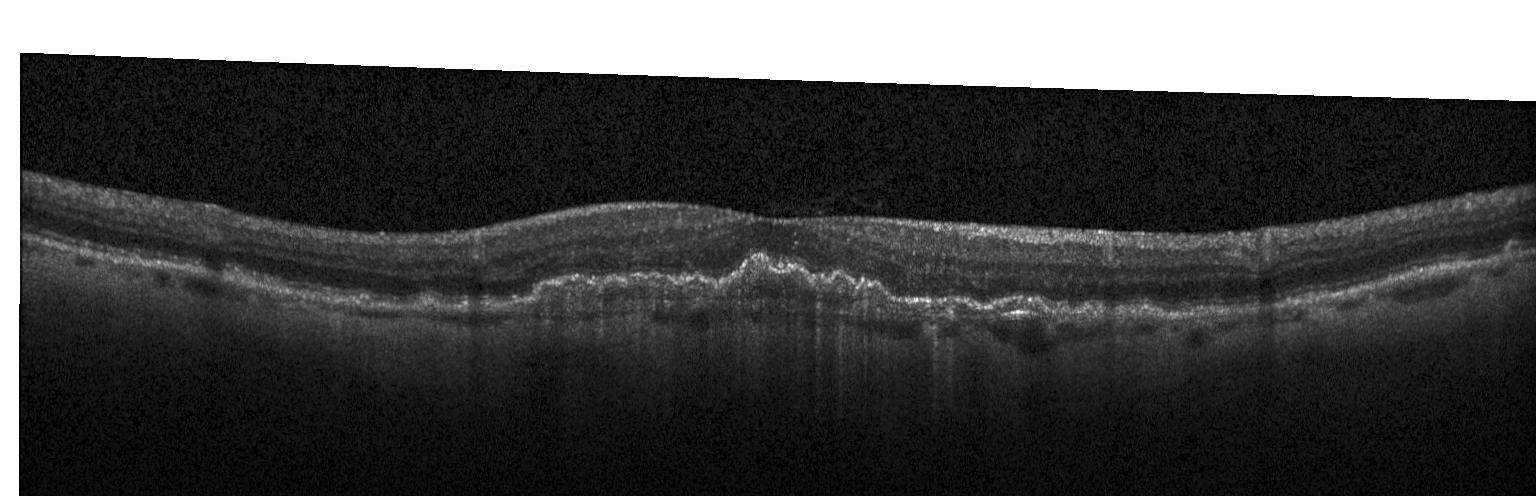 Impression: a choroidal neovascular membrane.